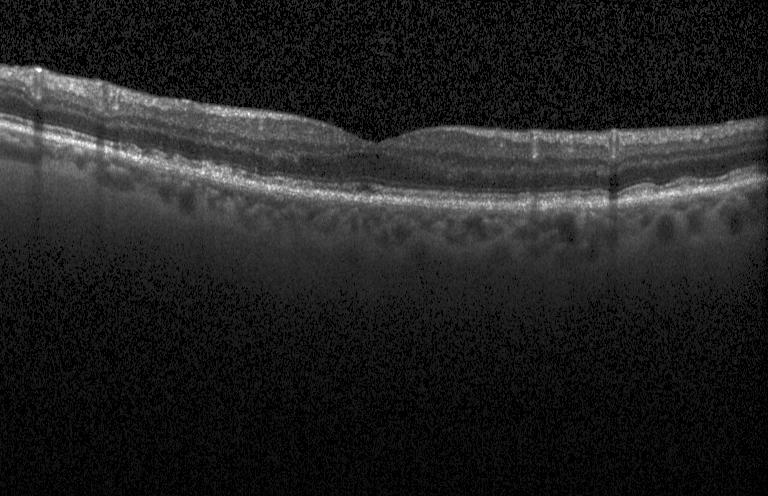
Spectral-domain OCT · OCT line scan.
Finding: drusen.